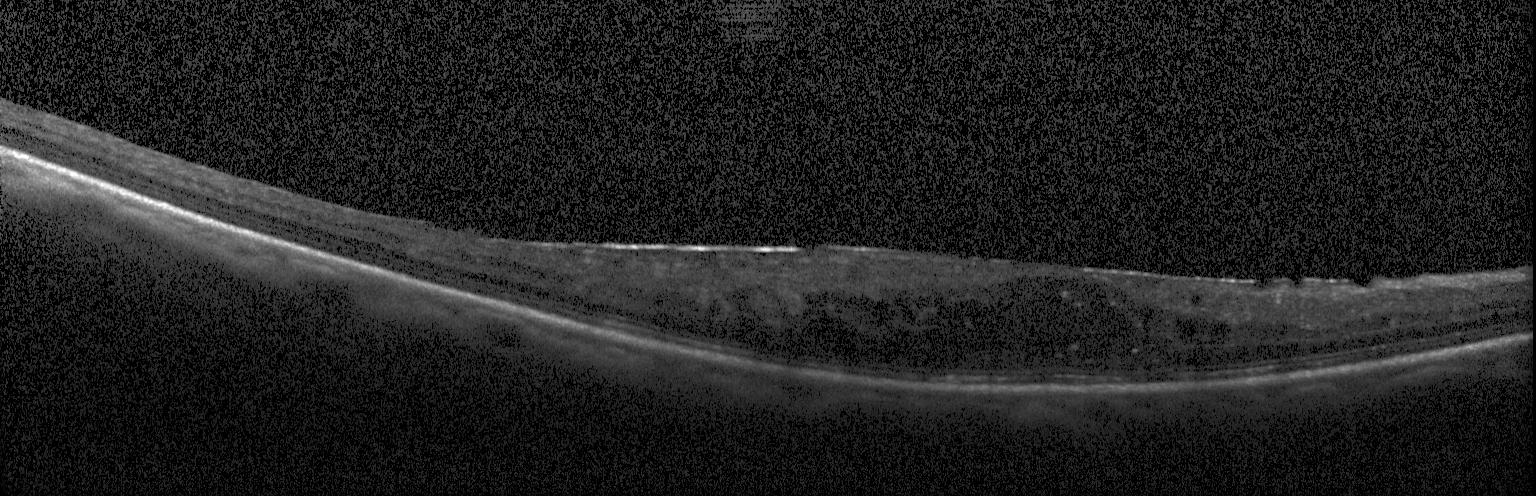 Finding: diabetic macular edema (DME).